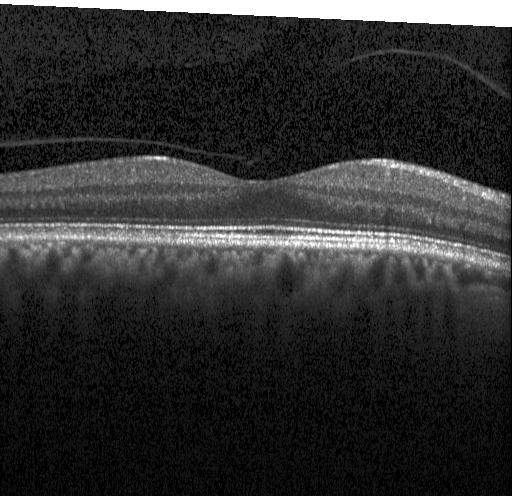
Horizontal scan through the fovea; instrument: Heidelberg Spectralis; OCT line scan.
Finding: no CNV, no DME, and no drusen.